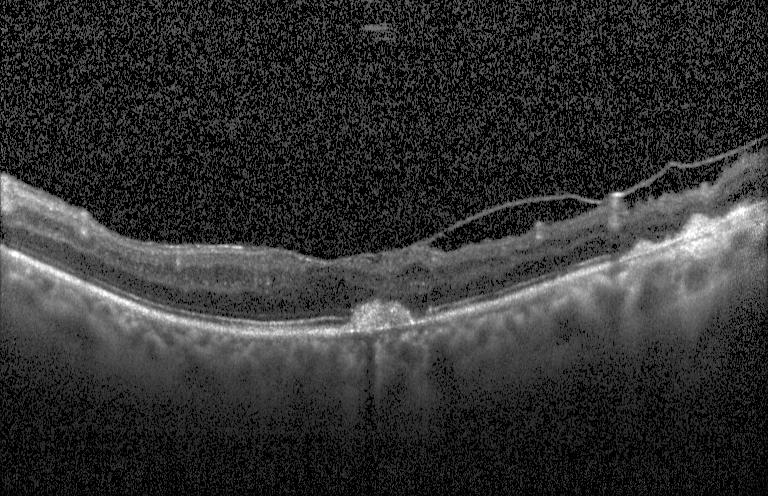
Fovea-centered; OCT B-scan; spectral-domain OCT. Finding: a choroidal neovascular membrane.